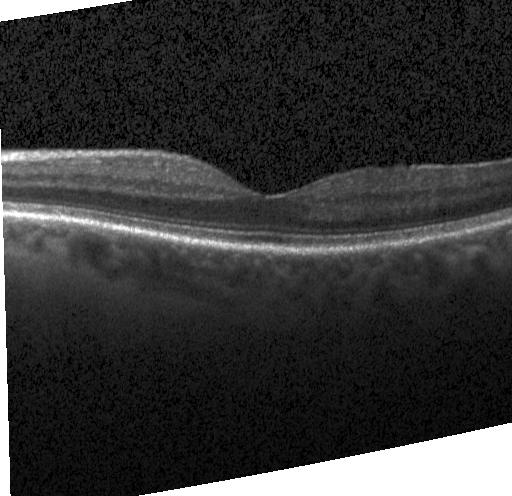
OCT line scan
Impression: no CNV, DME, or drusen.